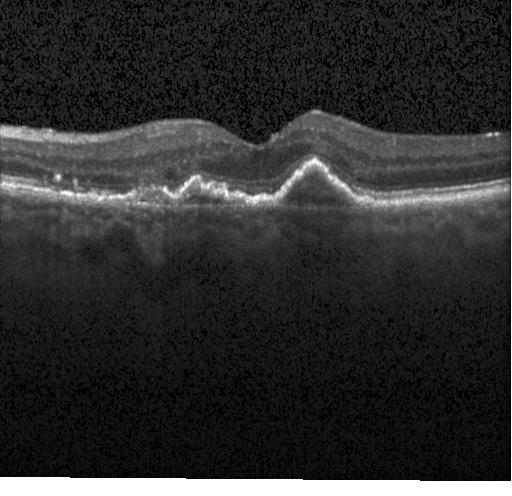

Instrument: Heidelberg Spectralis · OCT B-scan. Assessment: choroidal neovascularization.